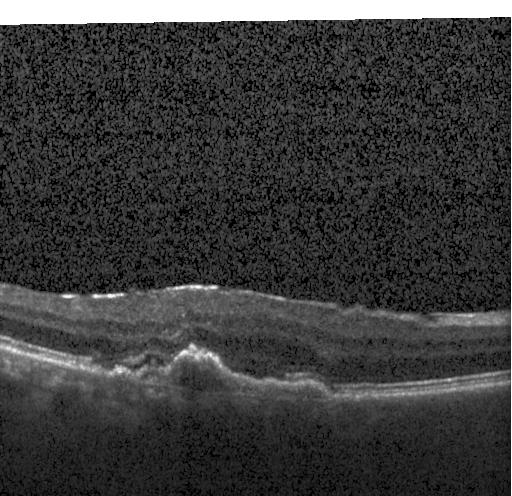 Finding: a choroidal neovascular membrane.